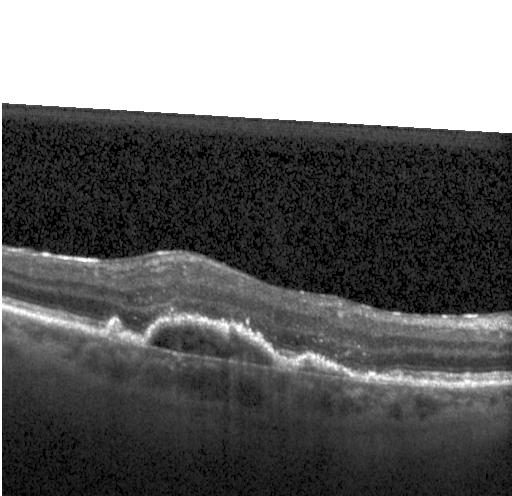

OCT B-scan; through the macula; instrument: Heidelberg Spectralis — Dx: a choroidal neovascular membrane.